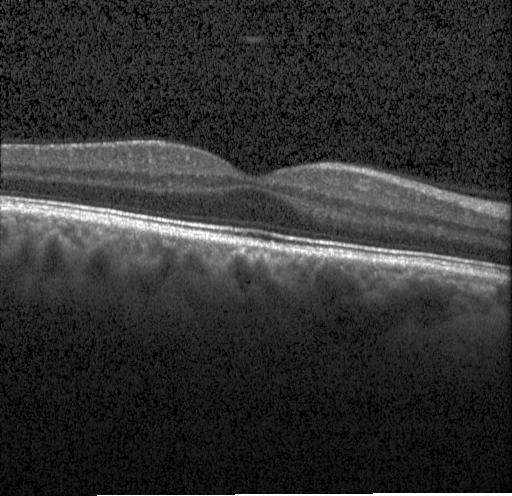
OCT line scan. OCT finding: no evidence of choroidal neovascularization, diabetic macular edema, or drusen.